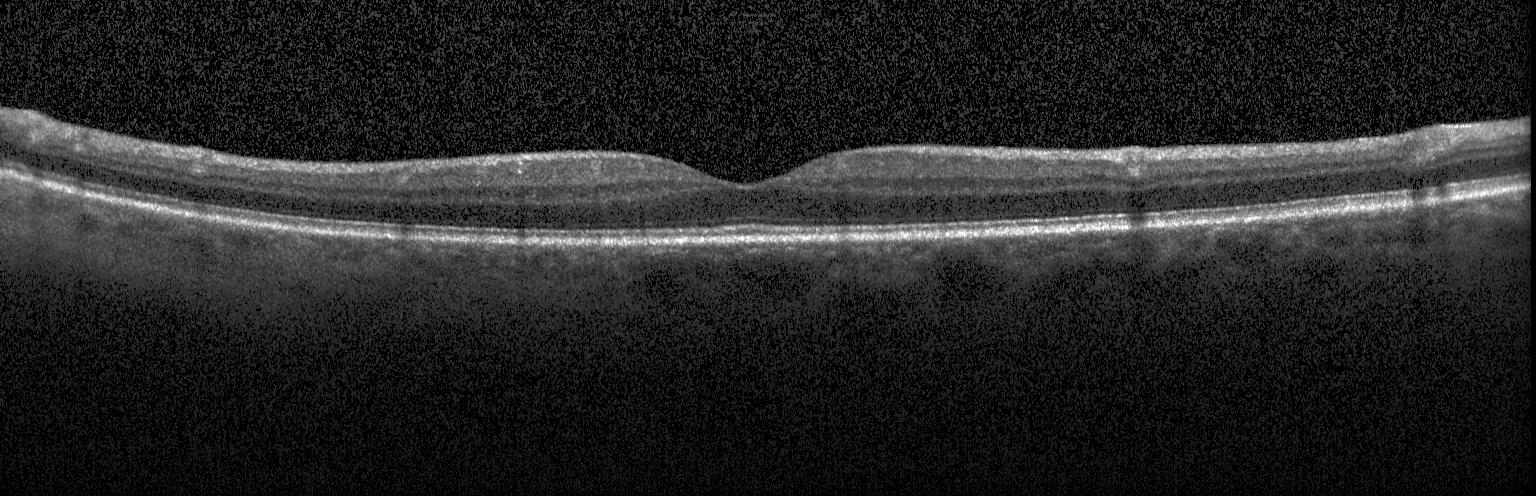

OCT B-scan. Finding: no choroidal neovascularization, no diabetic macular edema, and no drusen.